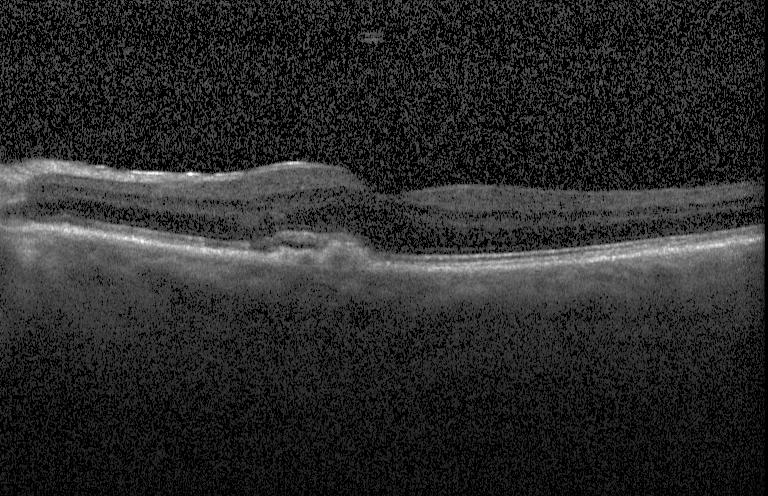
OCT finding: choroidal neovascularization (CNV).